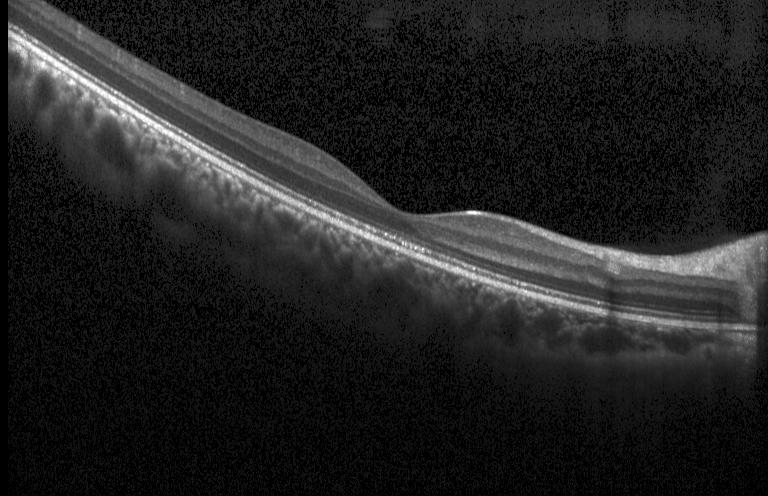 This B-scan demonstrates no choroidal neovascularization, diabetic macular edema, or drusen.